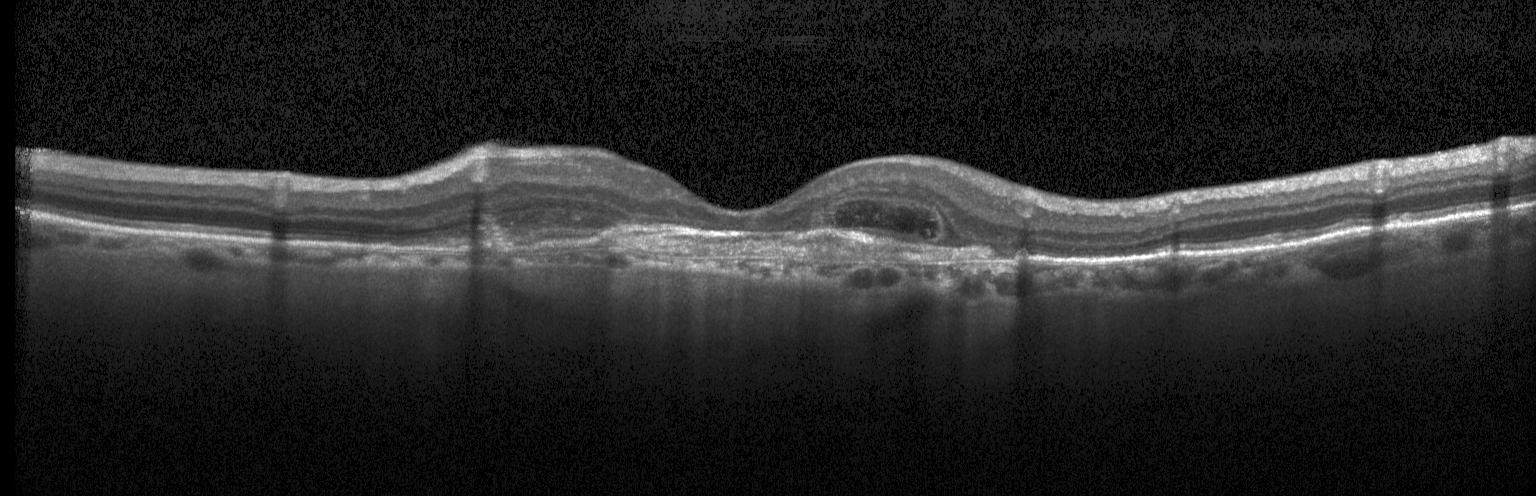
Heidelberg Spectralis OCT system; centered on the fovea; OCT B-scan; SD-OCT — Dx: choroidal neovascularization.